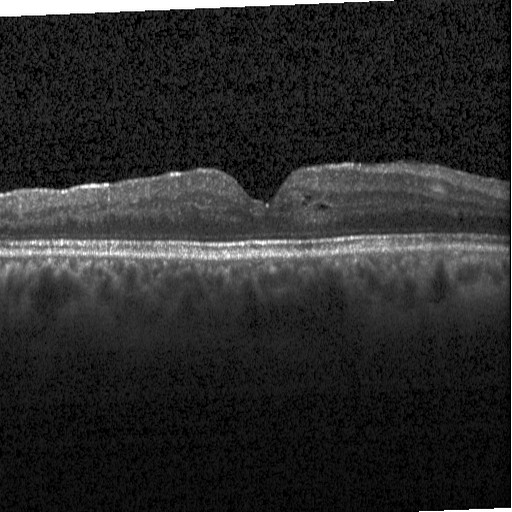
DME.